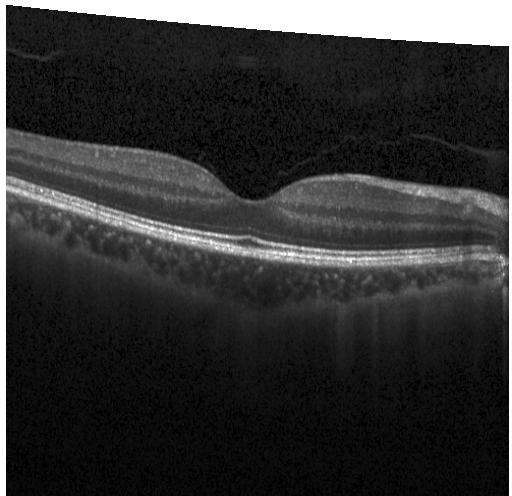
OCT line scan — This B-scan demonstrates no choroidal neovascularization, no diabetic macular edema, and no drusen.